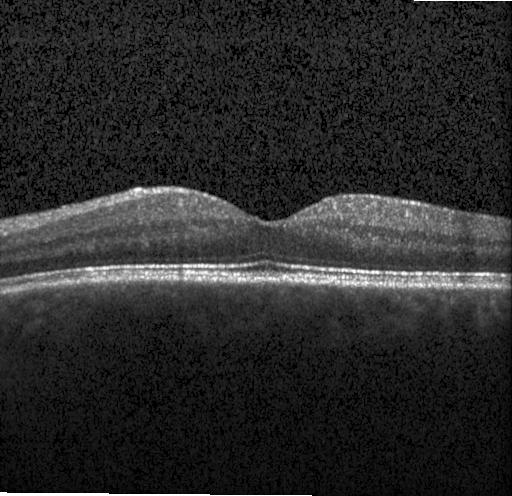
Finding: no evidence of choroidal neovascularization, diabetic macular edema, or drusen.